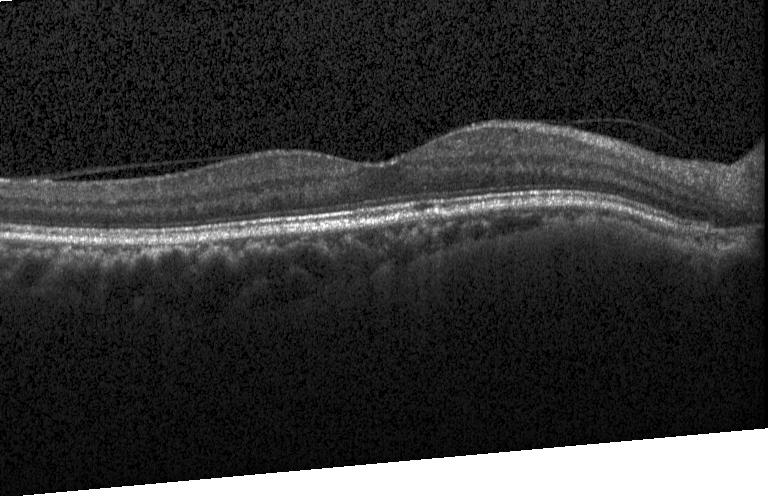 Acquired on a Heidelberg Spectralis · horizontal scan through the fovea · OCT line scan. Finding: no choroidal neovascularization, no diabetic macular edema, and no drusen.